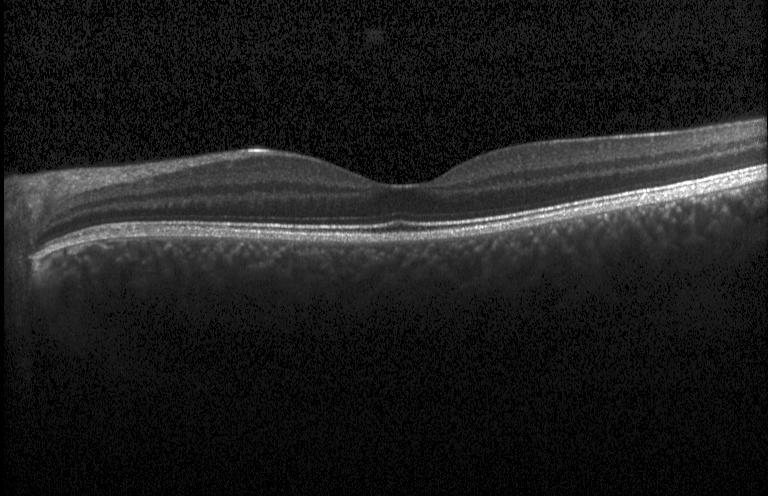
OCT line scan
Finding: no choroidal neovascularization, diabetic macular edema, or drusen.